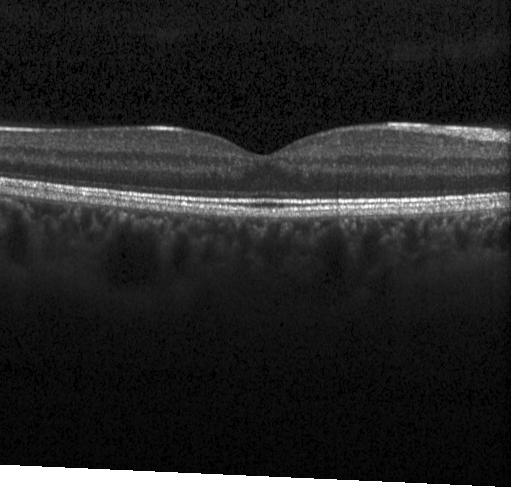 Retinal OCT cross-section, spectral-domain OCT, horizontal scan through the fovea
OCT finding: no evidence of CNV, DME, or drusen.